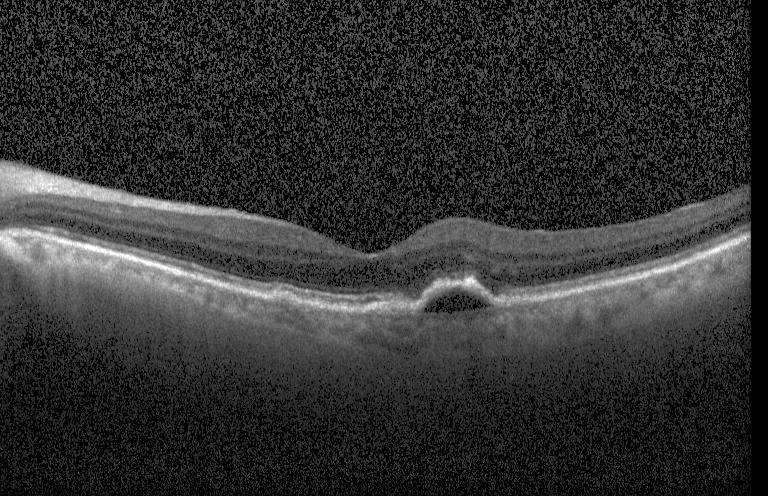
OCT B-scan.
The scan shows a choroidal neovascular membrane.